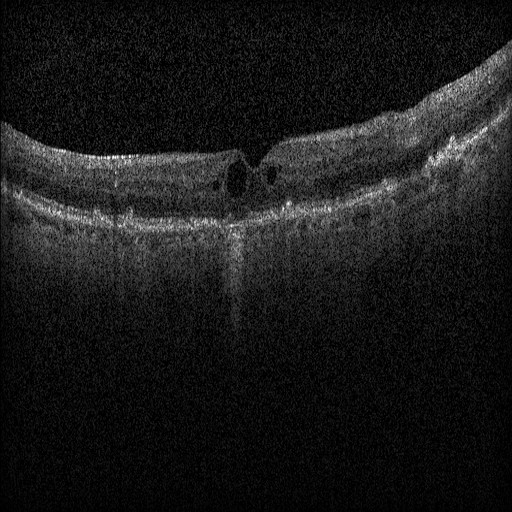
Spectral-domain OCT. Through the macula. Instrument: Heidelberg Spectralis. OCT B-scan
Assessment: DME.